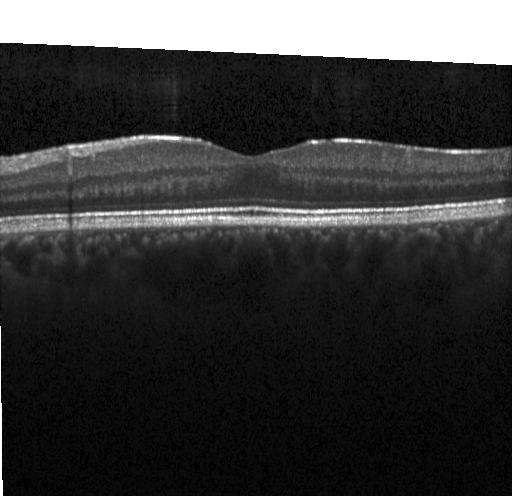

SD-OCT; acquired on a Heidelberg Spectralis; optical coherence tomography scan. Impression: no choroidal neovascularization, no diabetic macular edema, and no drusen.